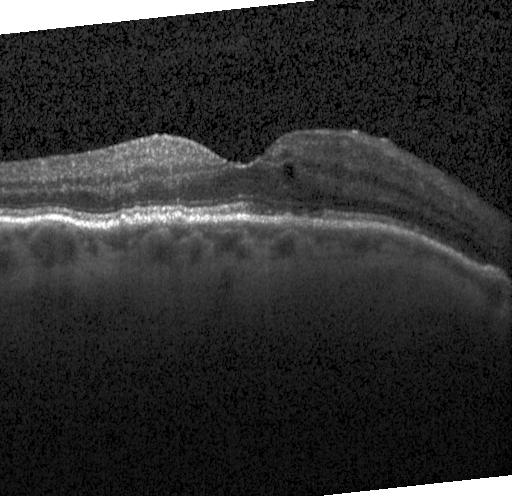
Heidelberg Spectralis, through the macula, spectral-domain OCT, OCT line scan — Choroidal neovascularization.